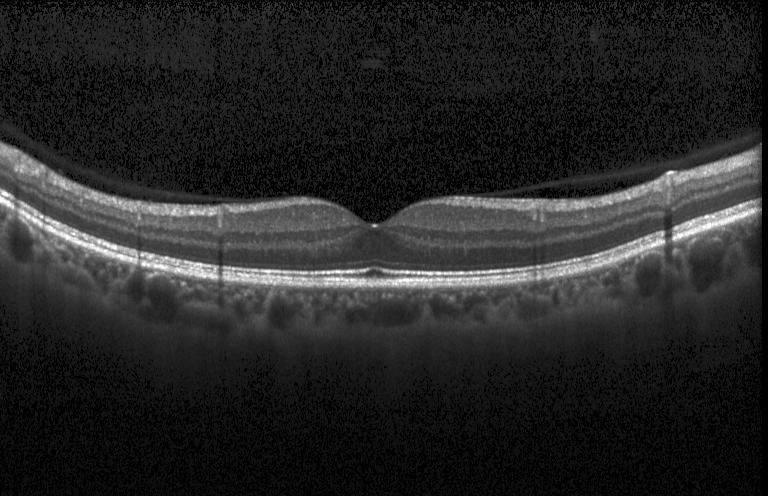

Finding: no choroidal neovascularization, diabetic macular edema, or drusen.